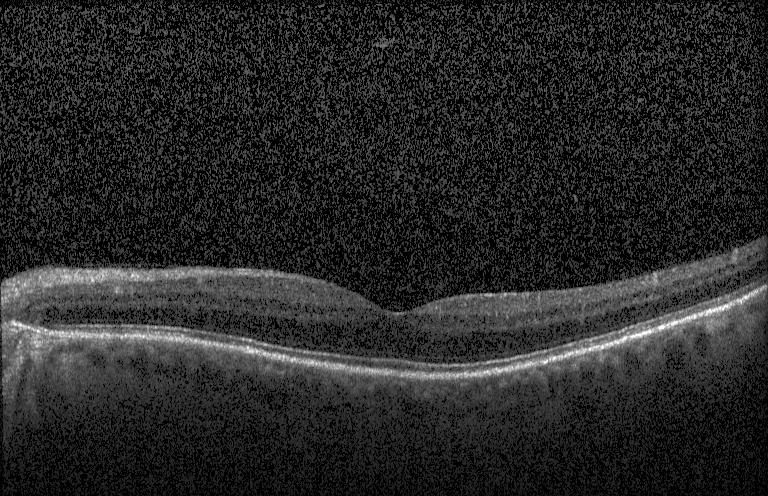

Spectral-domain optical coherence tomography, acquired on a Heidelberg Spectralis, optical coherence tomography scan, macular scan.
This B-scan demonstrates no CNV, no DME, and no drusen.